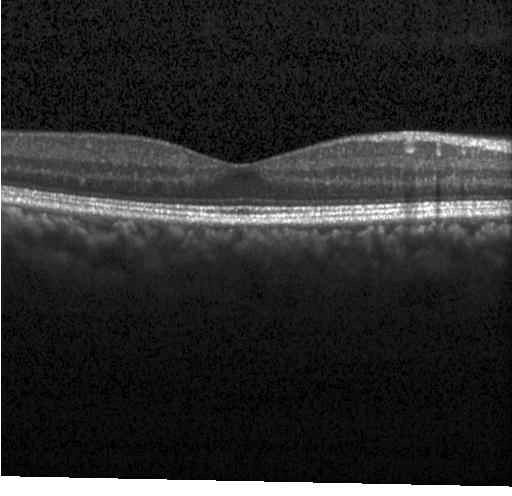 Diagnosis: no CNV, DME, or drusen.